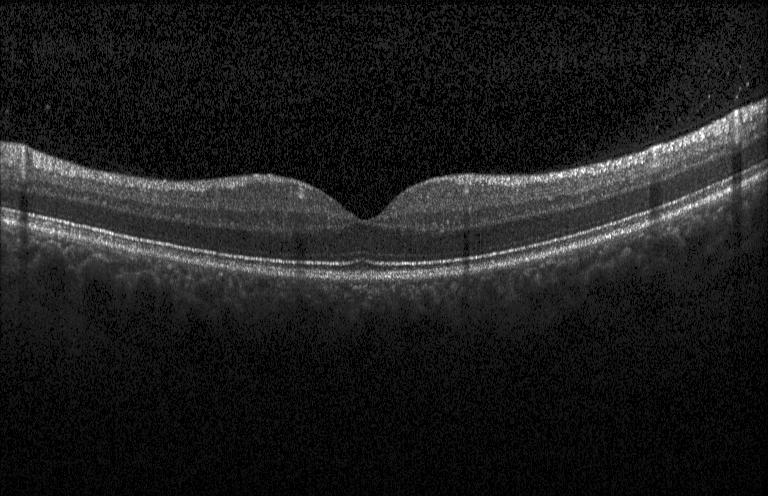
Assessment: no choroidal neovascularization, no diabetic macular edema, and no drusen.